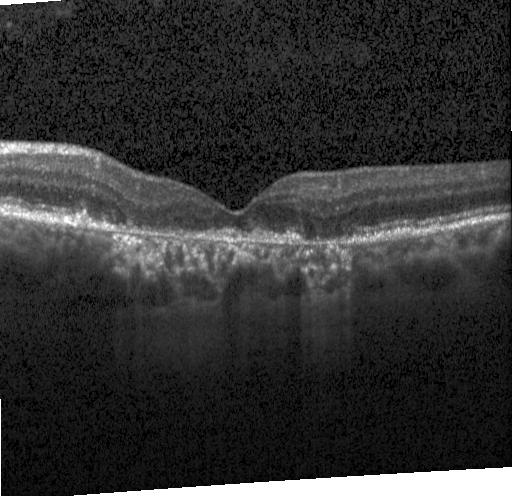

OCT B-scan. Diagnosis: a choroidal neovascular membrane.